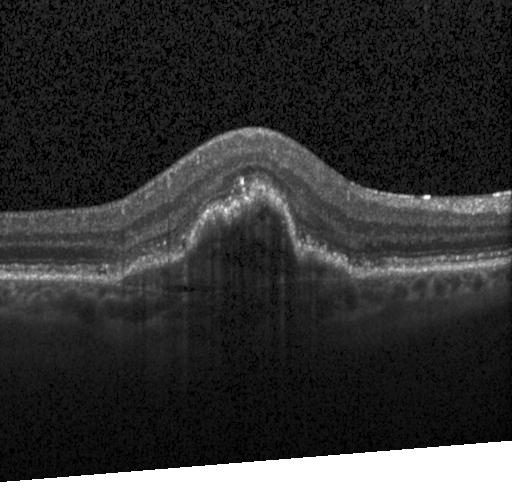

Optical coherence tomography scan — The scan shows a choroidal neovascular membrane.